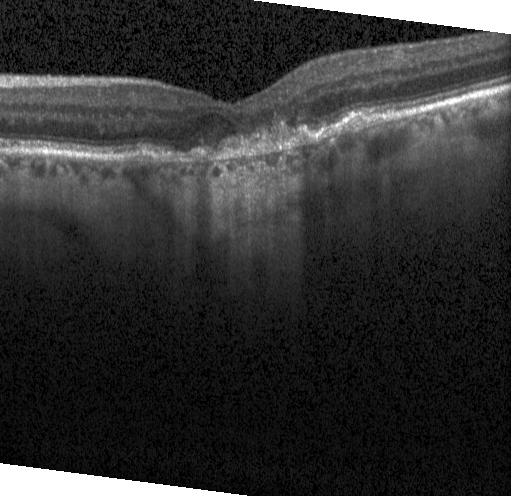
Spectral-domain optical coherence tomography; optical coherence tomography B-scan — Dx: a choroidal neovascular membrane.